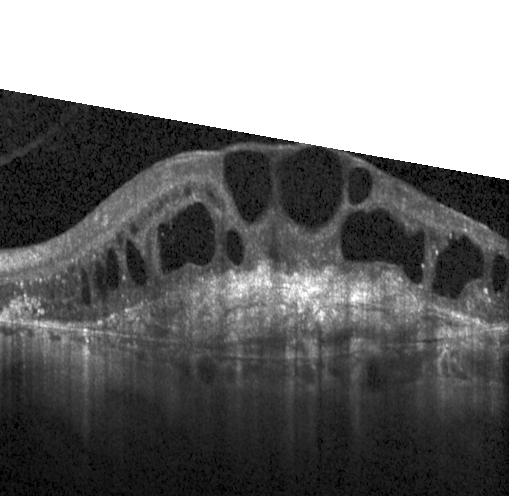 Heidelberg Spectralis OCT system, retinal OCT B-scan.
Diagnosis: choroidal neovascularization (CNV).